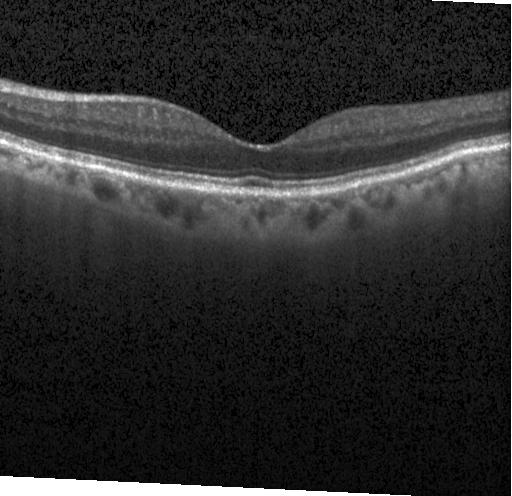
Diagnosis: no CNV, DME, or drusen.